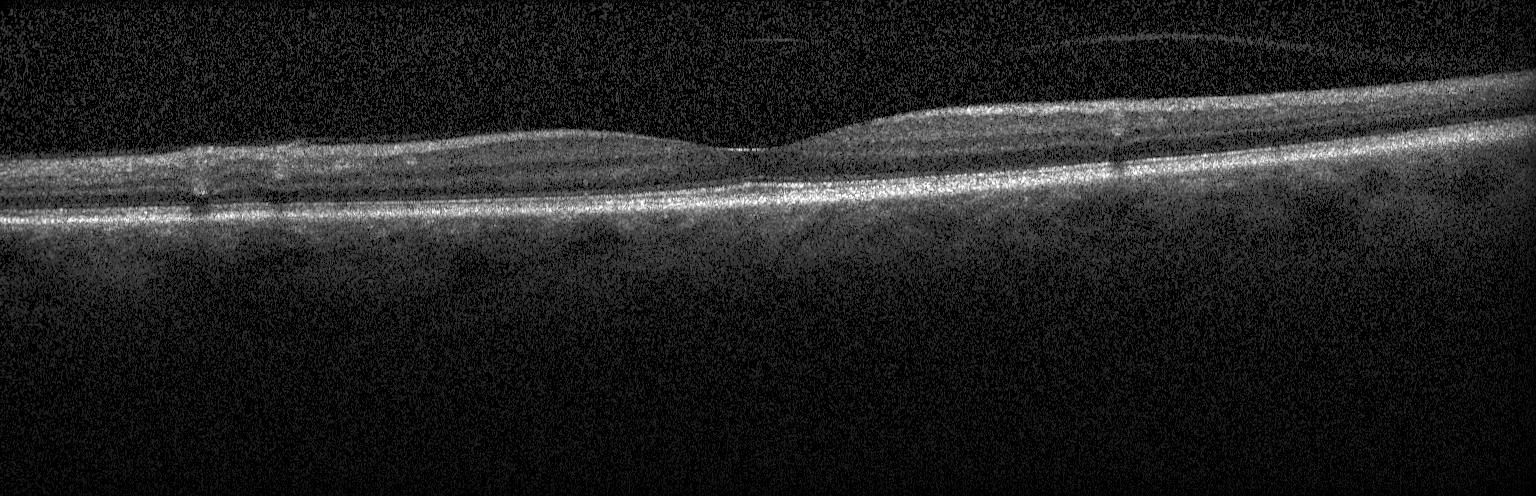
Heidelberg Spectralis, retinal OCT cross-section.
OCT finding: no choroidal neovascularization, no diabetic macular edema, and no drusen.